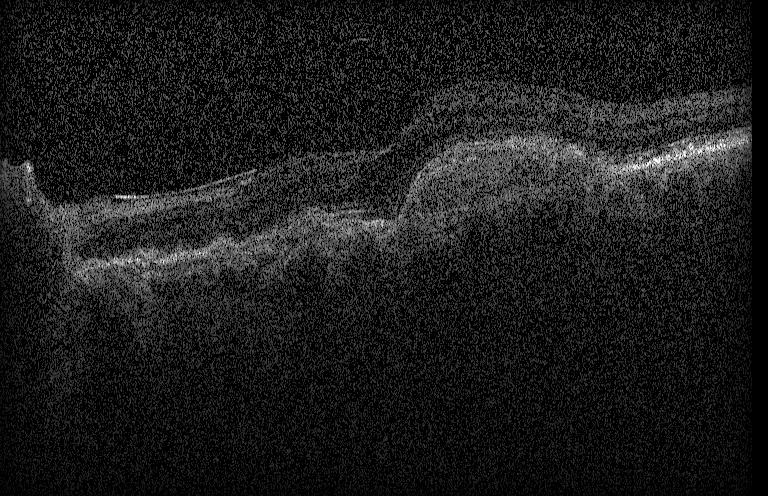 Diagnosis: choroidal neovascularization (CNV).